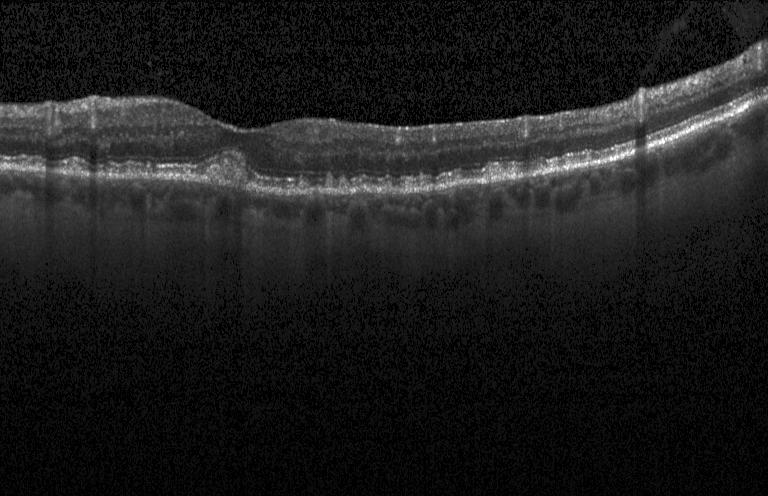

The scan shows multiple drusen.